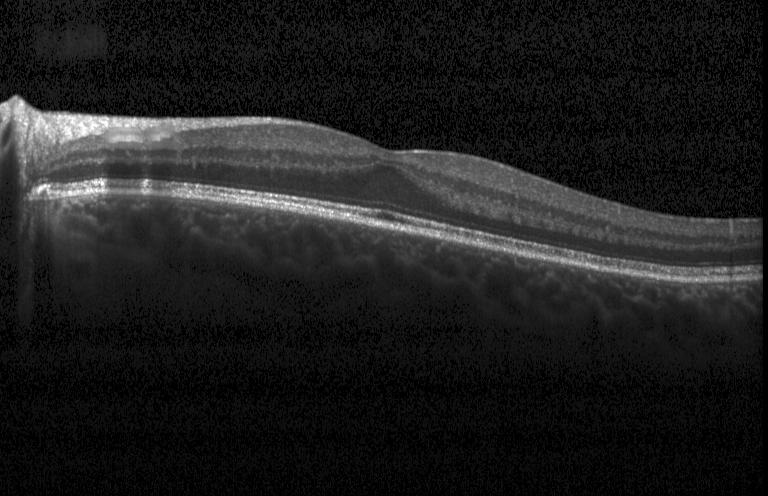
OCT line scan. Horizontal scan through the fovea. Spectral-domain optical coherence tomography. Instrument: Heidelberg Spectralis. Impression: no evidence of CNV, DME, or drusen.